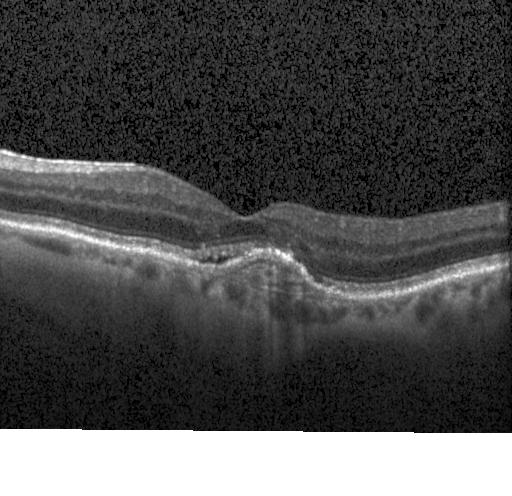

Spectral-domain optical coherence tomography · Heidelberg Spectralis · optical coherence tomography B-scan · through the macula. Diagnosis: a choroidal neovascular membrane.